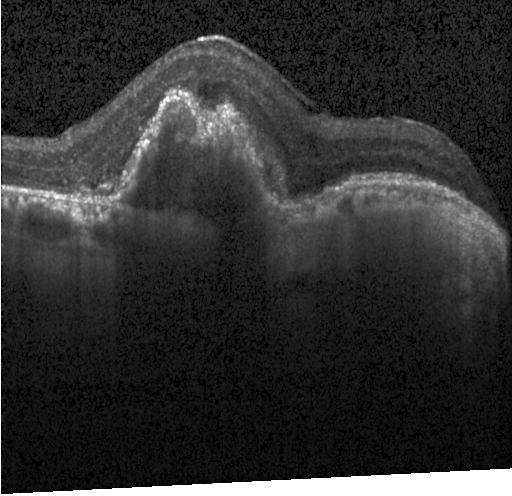 Optical coherence tomography B-scan; instrument: Heidelberg Spectralis; macular scan — Diagnosis: a choroidal neovascular membrane.